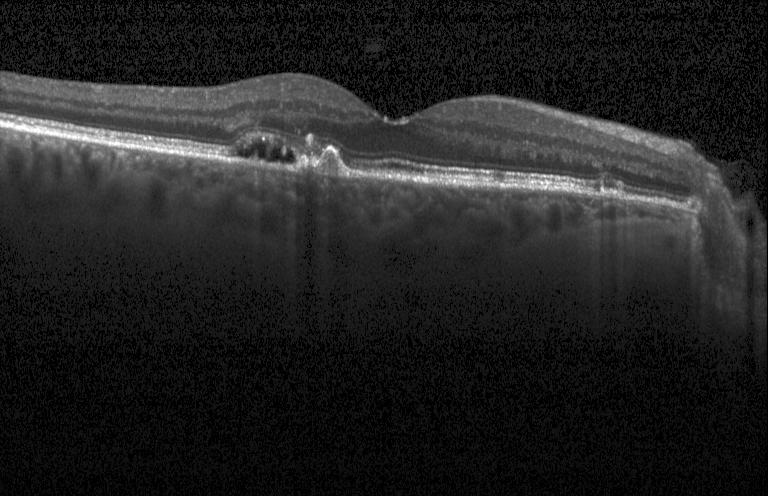 Retinal OCT cross-section.
Diagnosis: a choroidal neovascular membrane.